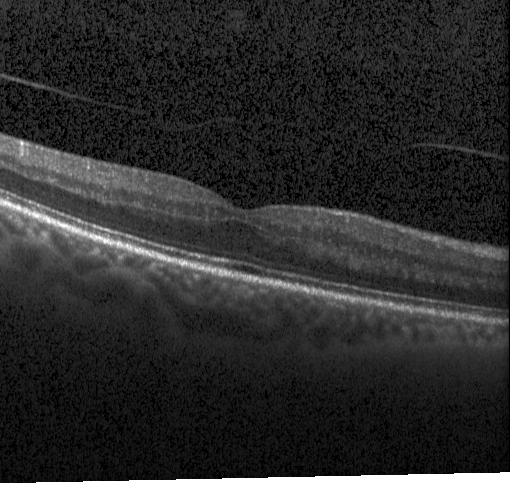
Optical coherence tomography scan — The scan shows no evidence of choroidal neovascularization, diabetic macular edema, or drusen.